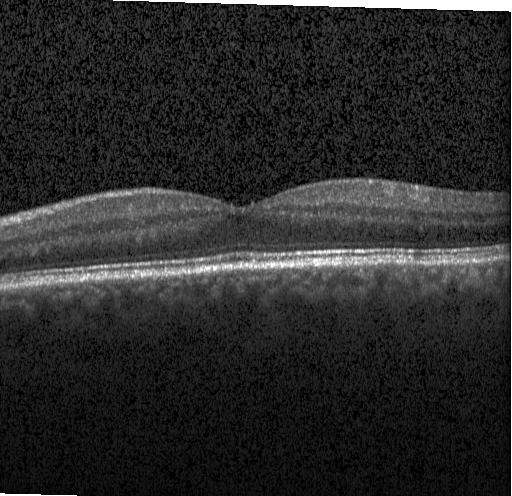
OCT finding: neither choroidal neovascularization, diabetic macular edema, nor drusen.